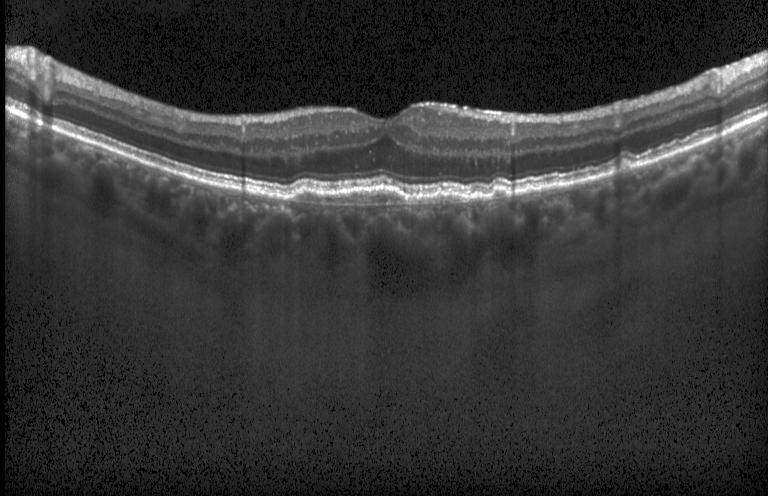 Optical coherence tomography B-scan
Dx: choroidal neovascularization (CNV).